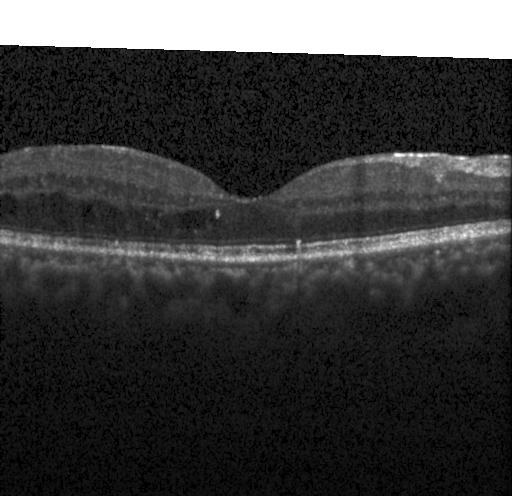 Spectral-domain OCT; acquired on a Heidelberg Spectralis; optical coherence tomography scan; fovea-centered — Assessment: diabetic macular edema.